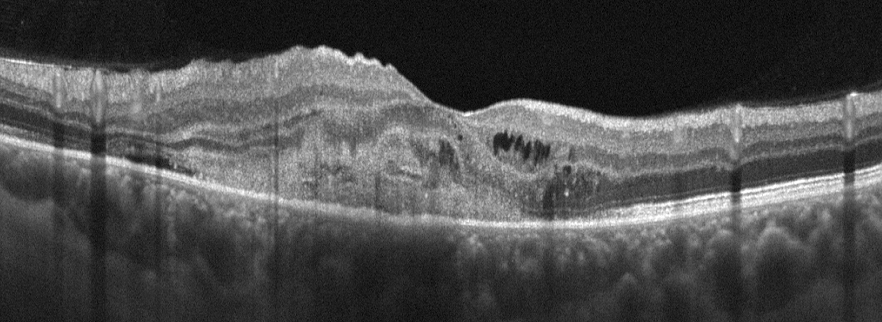
Oculus dexter, retinal OCT cross-section.
Impression: AMD.